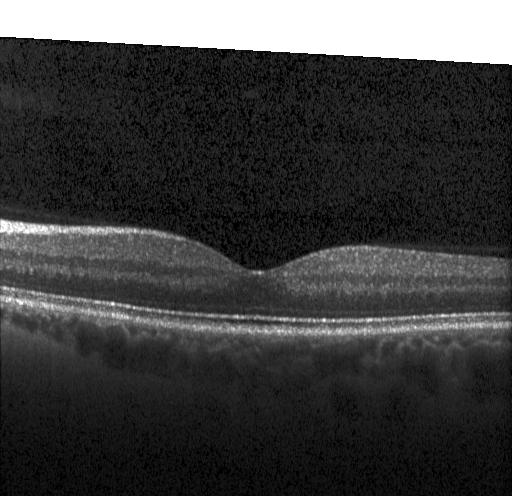 Retinal OCT cross-section showing no evidence of choroidal neovascularization, diabetic macular edema, or drusen.